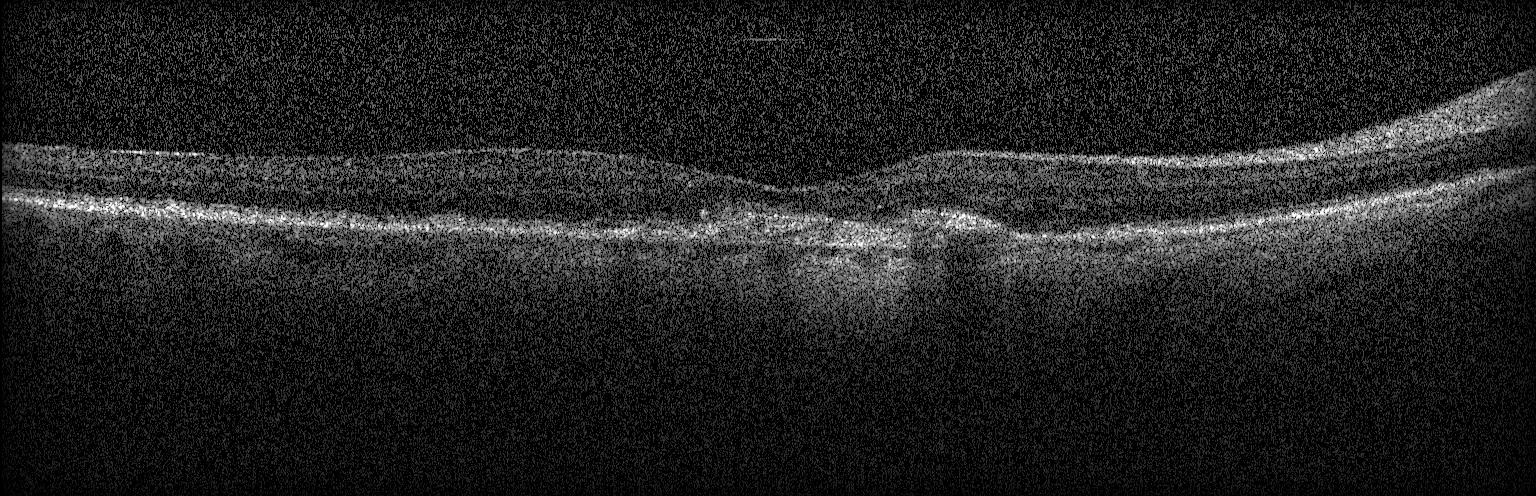

Retinal OCT cross-section.
OCT finding: a choroidal neovascular membrane.